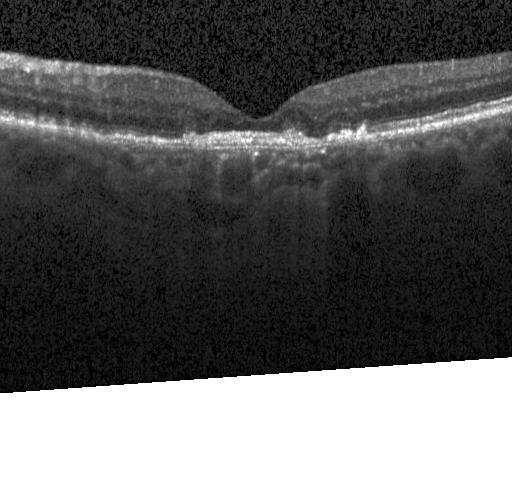
OCT B-scan showing CNV.